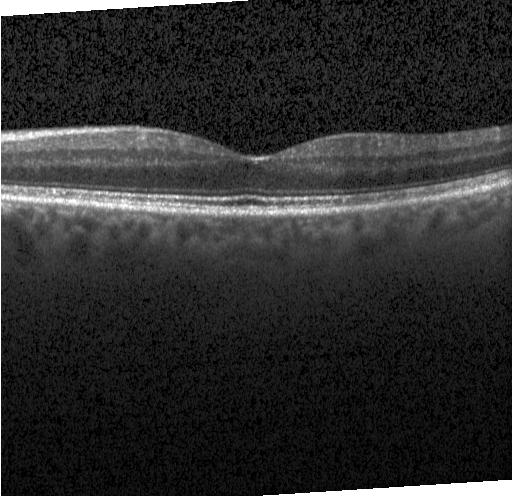

Retinal OCT cross-section. Heidelberg Spectralis OCT system.
OCT finding: no choroidal neovascularization, no diabetic macular edema, and no drusen.